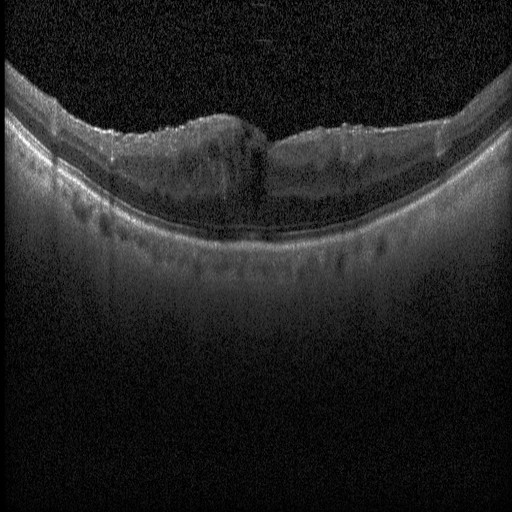
Optical coherence tomography B-scan
Assessment: diabetic macular edema.